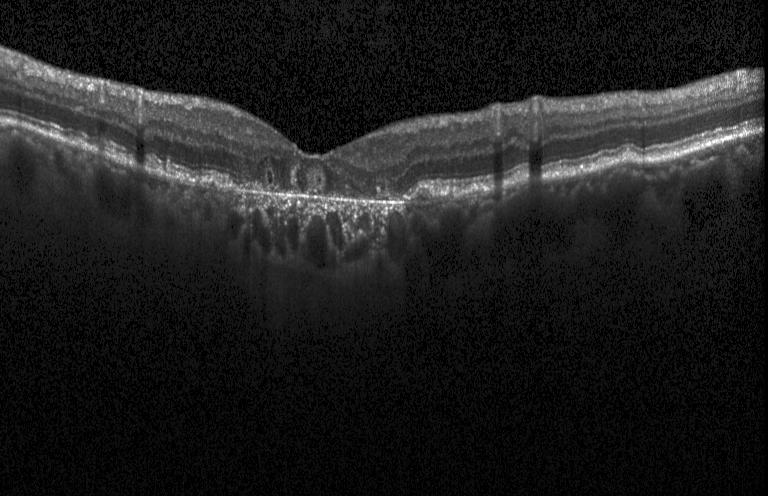
Heidelberg Spectralis OCT system · horizontal scan through the fovea · retinal OCT cross-section — Impression: choroidal neovascularization.